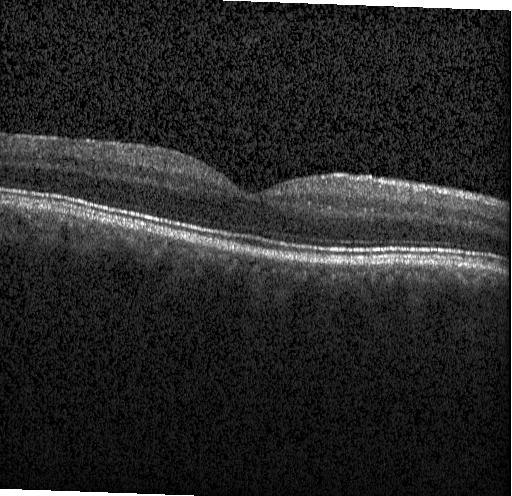 SD-OCT. OCT B-scan. Through the macula.
This B-scan demonstrates neither choroidal neovascularization, diabetic macular edema, nor drusen.